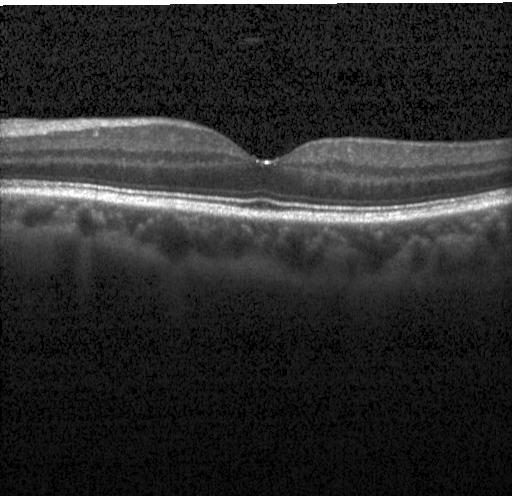 Spectral-domain optical coherence tomography, retinal OCT cross-section, instrument: Heidelberg Spectralis, through the macula — The scan shows no choroidal neovascularization, no diabetic macular edema, and no drusen.